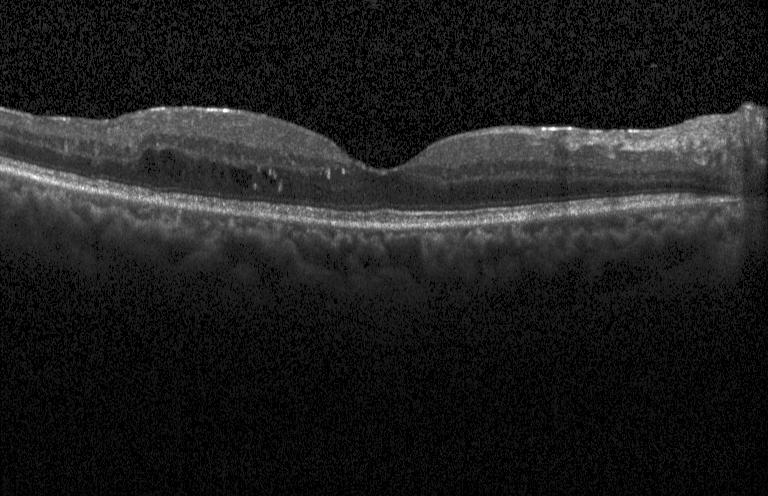 Spectral-domain OCT B-scan: diabetic macular edema.